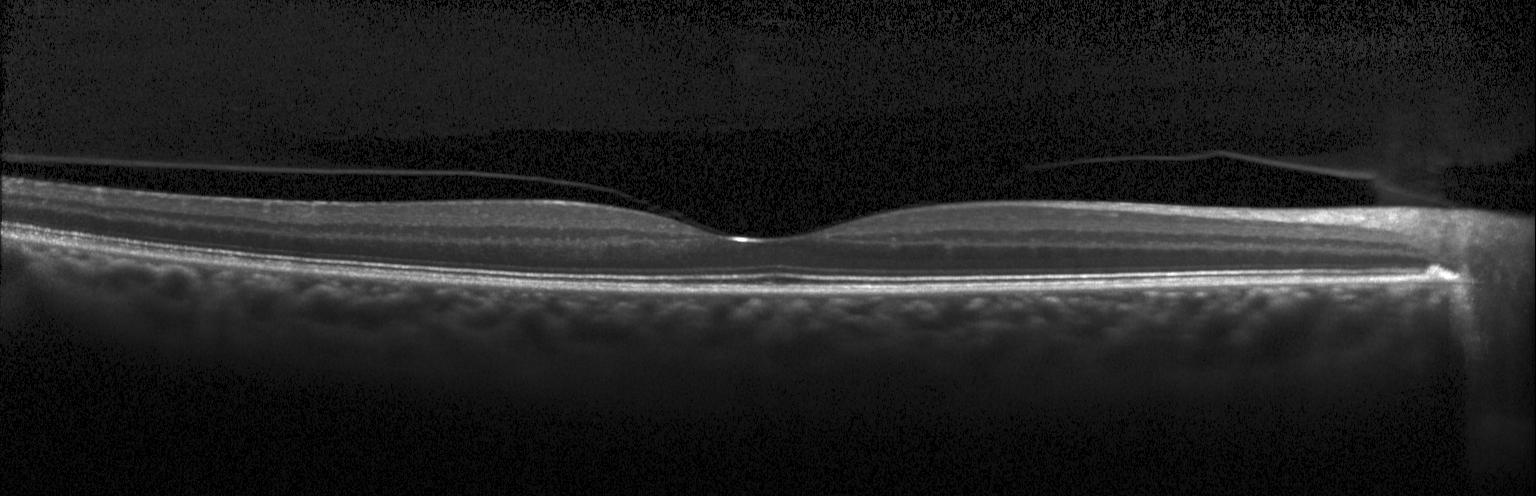
Macular scan. OCT B-scan. Spectral-domain optical coherence tomography. Acquired on a Heidelberg Spectralis
Impression: no CNV, DME, or drusen.